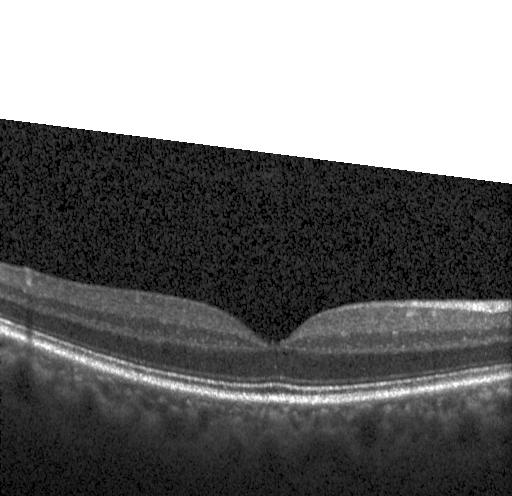

OCT B-scan; SD-OCT. OCT finding: neither choroidal neovascularization, diabetic macular edema, nor drusen.